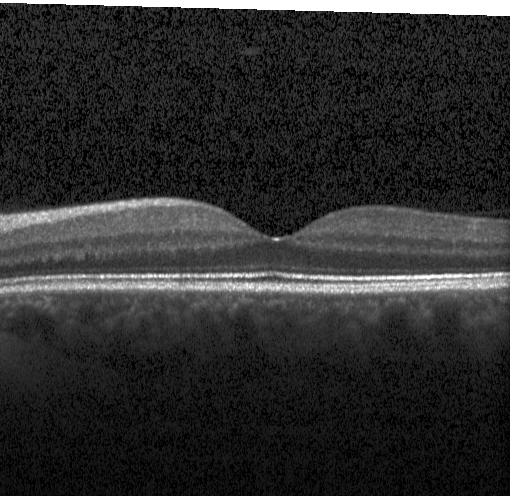
Impression: no evidence of choroidal neovascularization, diabetic macular edema, or drusen.